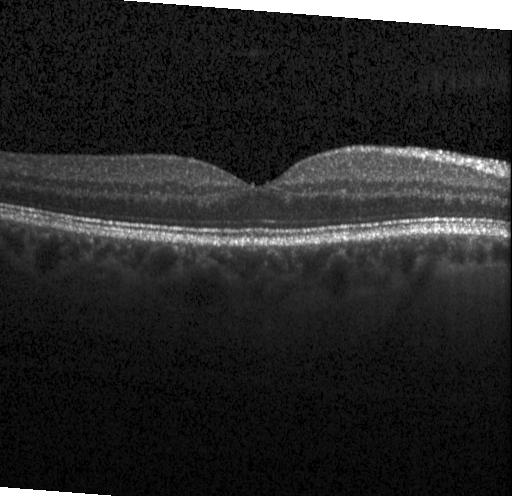

OCT scan showing neither choroidal neovascularization, diabetic macular edema, nor drusen.